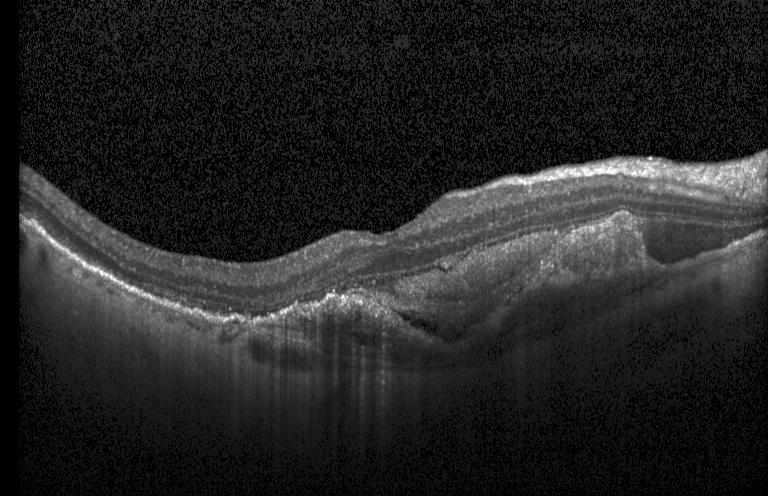
Finding: choroidal neovascularization (CNV).